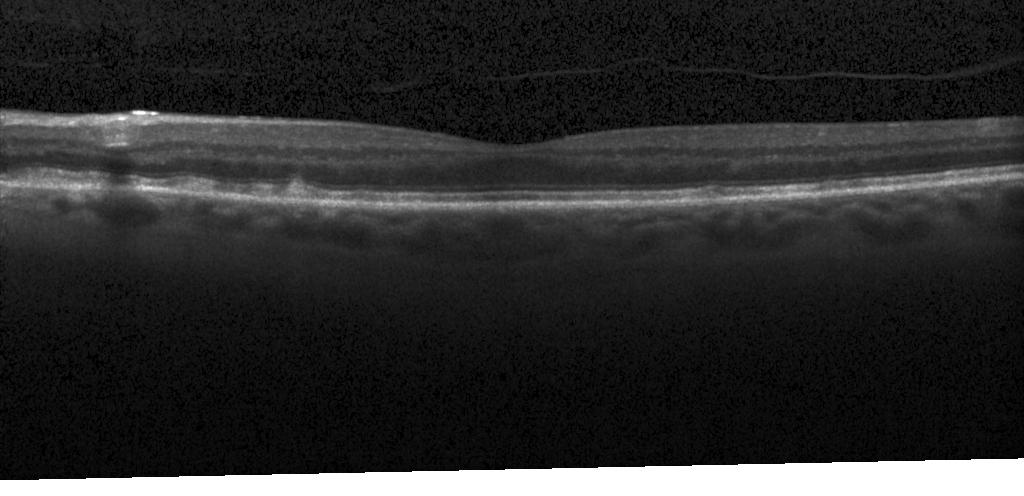
SD-OCT · optical coherence tomography scan · Heidelberg Spectralis.
Diagnosis: multiple drusen.